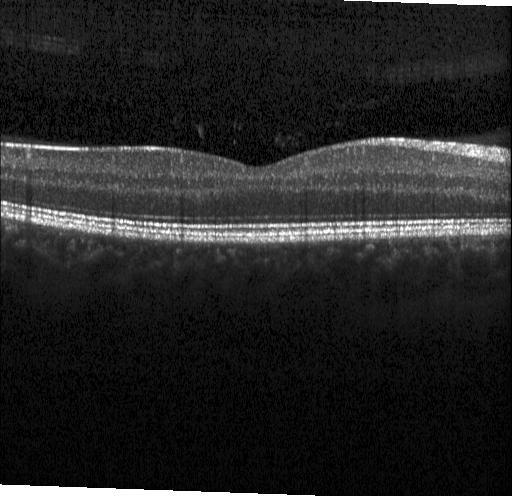 Macular OCT demonstrating no CNV, DME, or drusen.